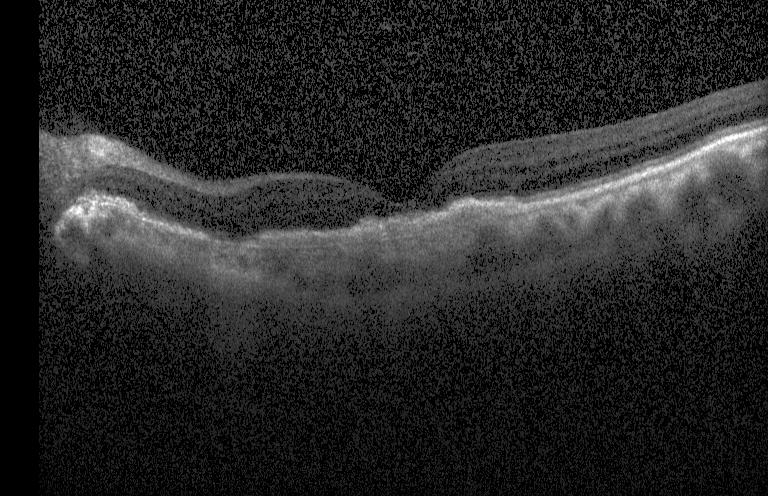

Optical coherence tomography B-scan; centered on the fovea. Macular OCT: choroidal neovascularization.